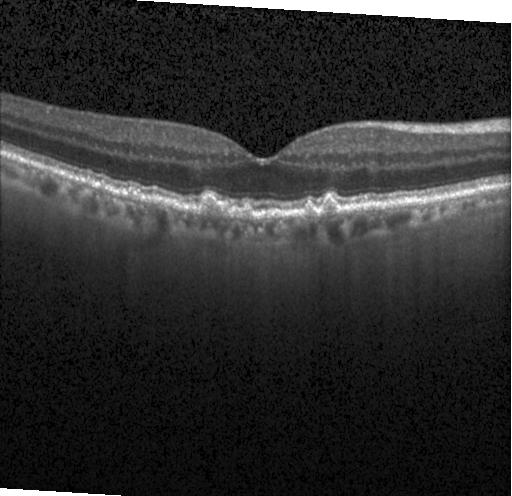

Dx: drusen.